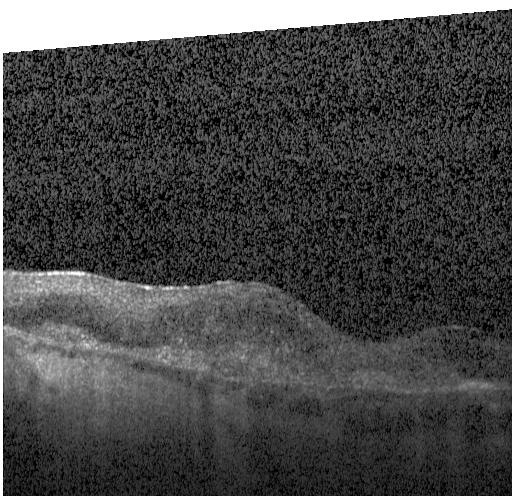 Retinal OCT cross-section showing CNV.